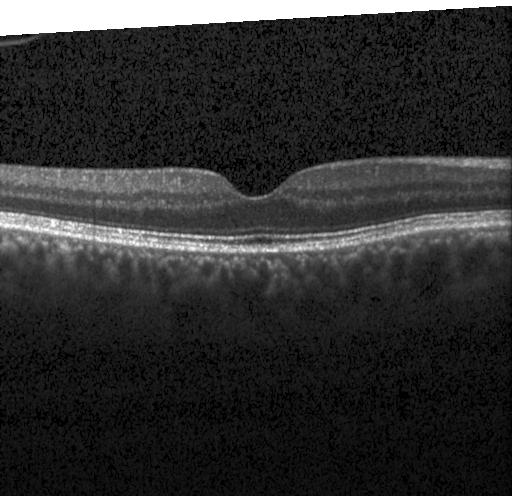

OCT B-scan — Diagnosis: no CNV, no DME, and no drusen.